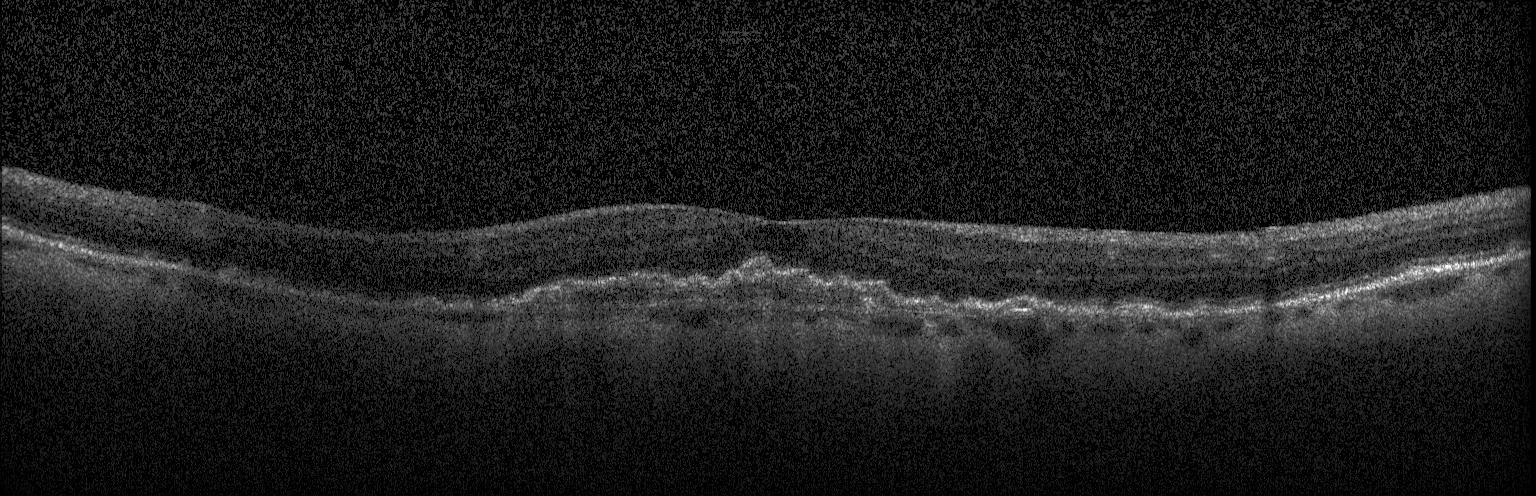
CNV.